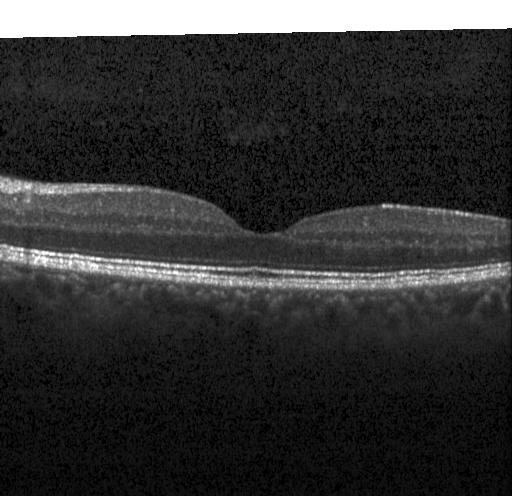 OCT finding: no choroidal neovascularization, no diabetic macular edema, and no drusen.